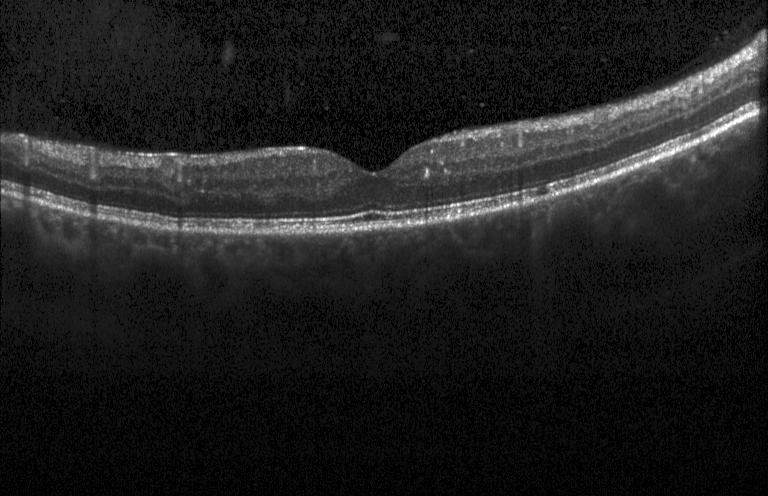 Retinal OCT cross-section showing no choroidal neovascularization, no diabetic macular edema, and no drusen.